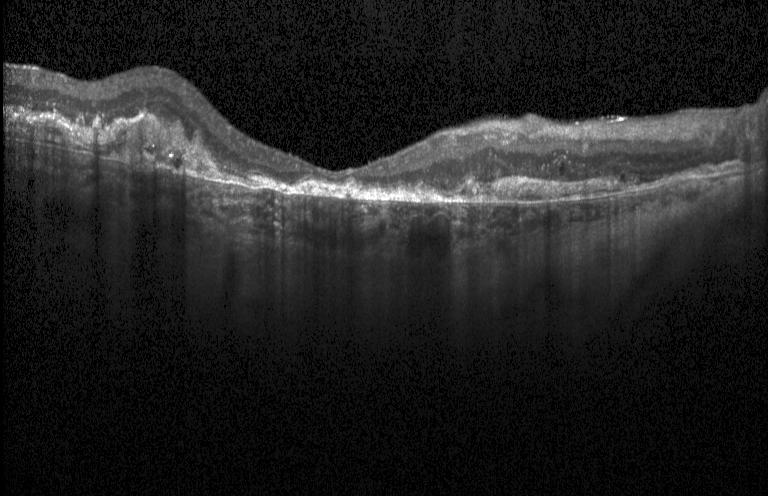
Optical coherence tomography scan. Fovea-centered. Spectral-domain OCT. Acquired on a Heidelberg Spectralis
Diagnosis: a choroidal neovascular membrane.